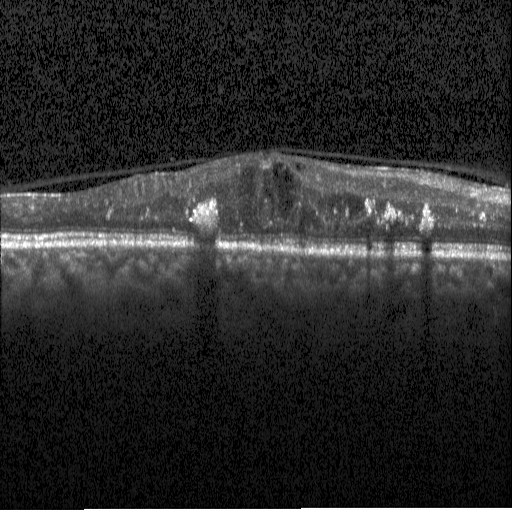 Through the macula, OCT B-scan.
Macular OCT: diabetic macular edema (DME).